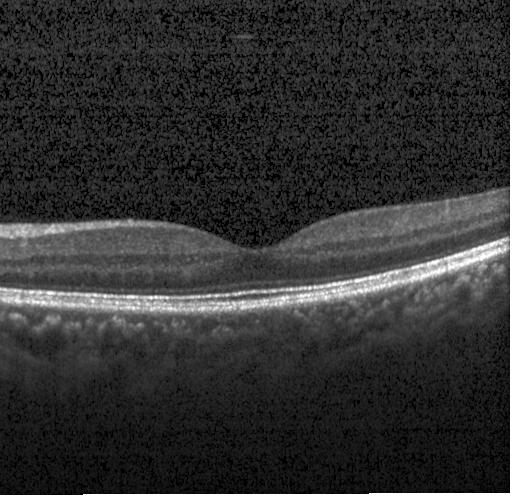

Heidelberg Spectralis OCT system, optical coherence tomography B-scan.
The scan shows no choroidal neovascularization, no diabetic macular edema, and no drusen.